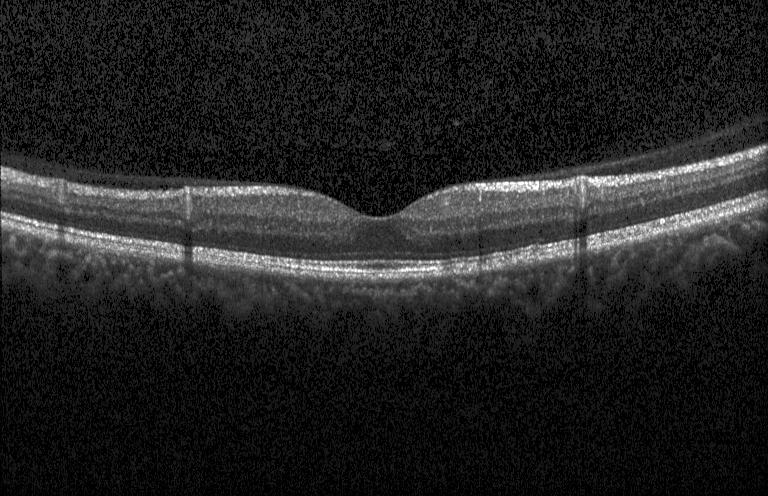 Through the macula · OCT line scan · SD-OCT · Heidelberg Spectralis. Macular OCT: no evidence of choroidal neovascularization, diabetic macular edema, or drusen.